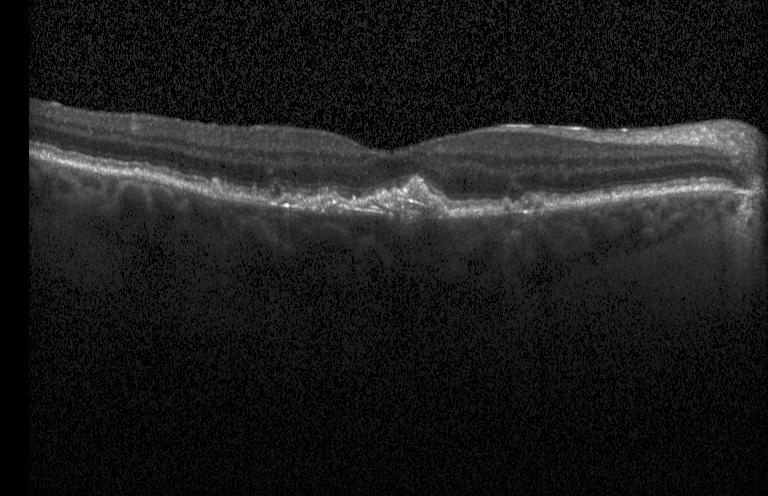
Optical coherence tomography scan; spectral-domain OCT — Assessment: a choroidal neovascular membrane.